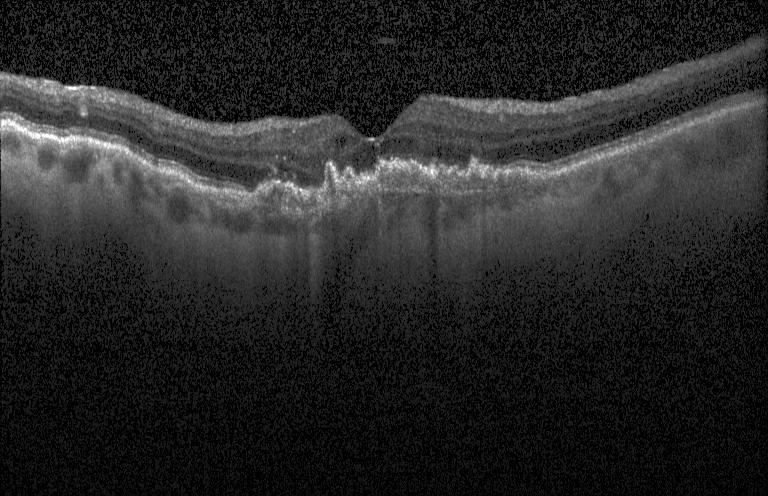 Heidelberg Spectralis. Optical coherence tomography B-scan — Finding: choroidal neovascularization (CNV).